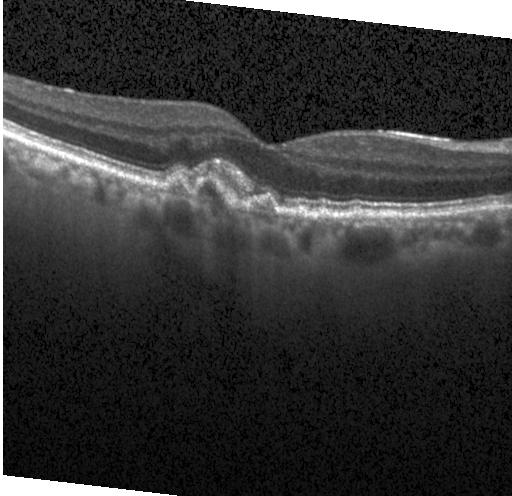

Assessment: a choroidal neovascular membrane.